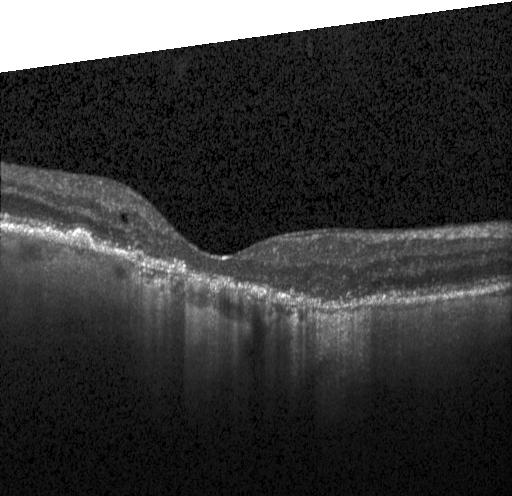

Optical coherence tomography B-scan, centered on the fovea. Finding: a choroidal neovascular membrane.